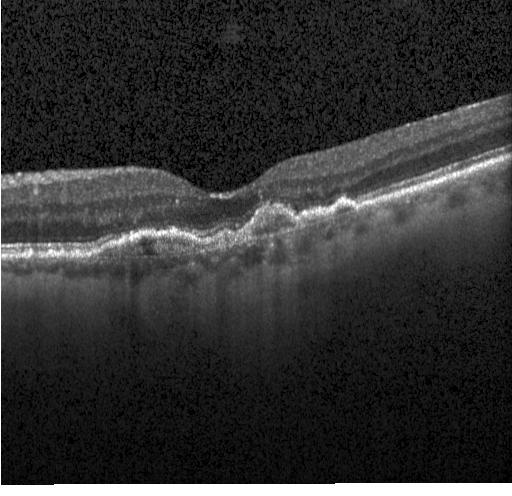

SD-OCT. Optical coherence tomography B-scan. Acquired on a Heidelberg Spectralis. Horizontal scan through the fovea.
Impression: choroidal neovascularization (CNV).